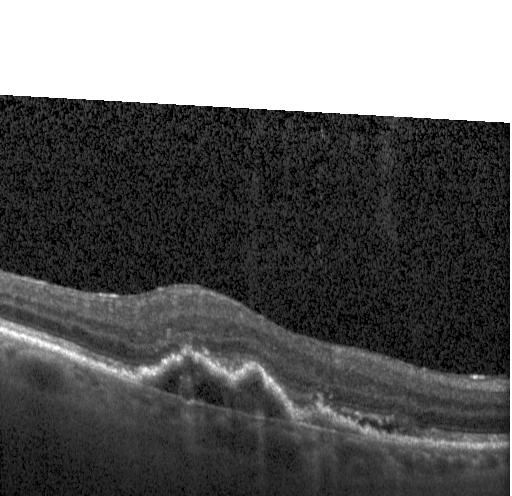 Impression: a choroidal neovascular membrane.